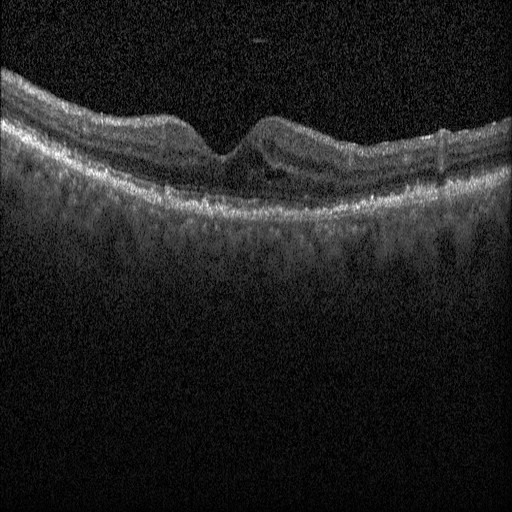

Macular OCT demonstrating DME.